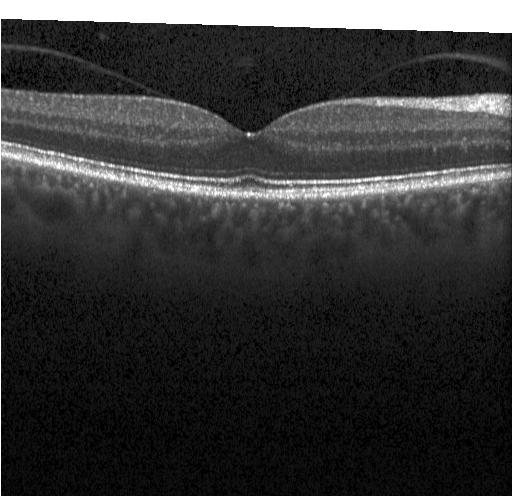

Diagnosis: no choroidal neovascularization, no diabetic macular edema, and no drusen.